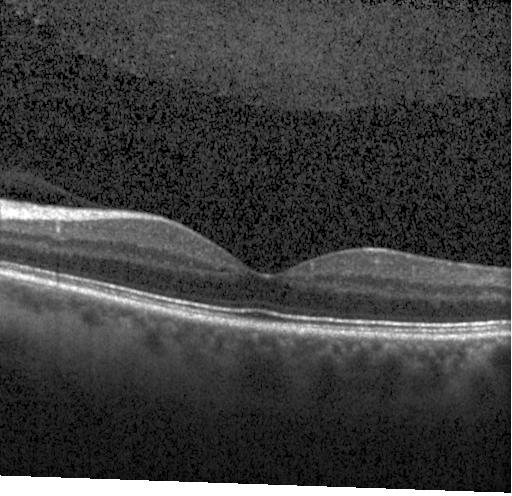

OCT B-scan showing neither CNV, DME, nor drusen.